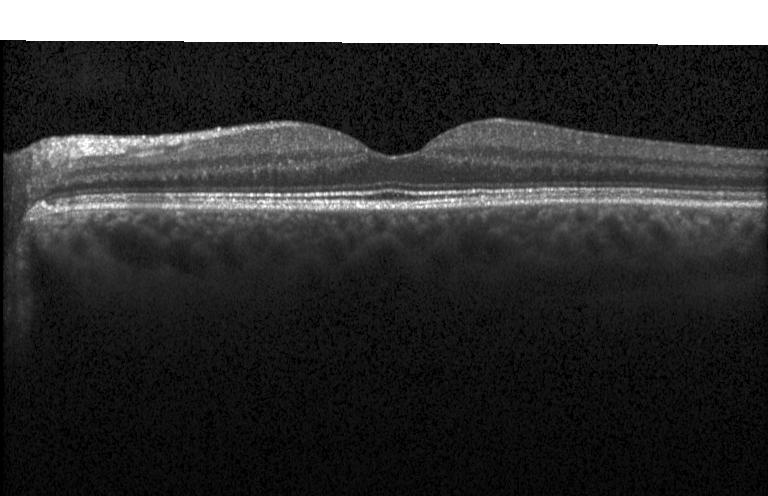
Instrument: Heidelberg Spectralis, retinal OCT cross-section, spectral-domain OCT, horizontal scan through the fovea
Macular OCT: neither CNV, DME, nor drusen.